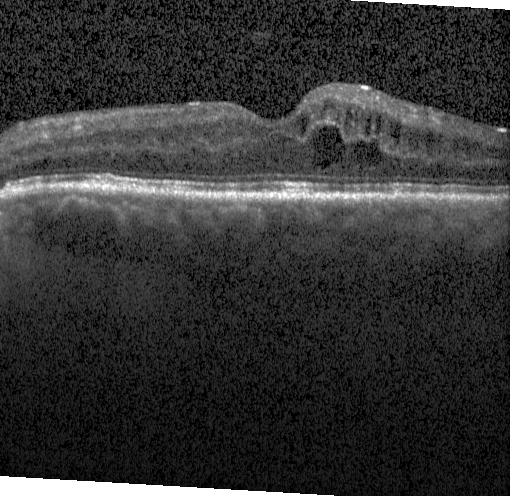
Finding: DME.